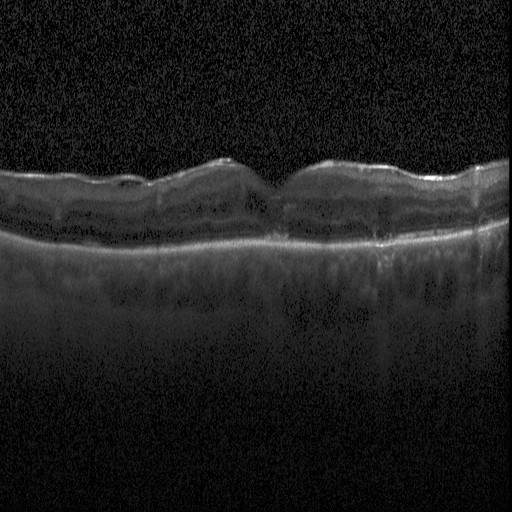 SD-OCT. Acquired on a Heidelberg Spectralis. OCT B-scan — Macular OCT: DME.